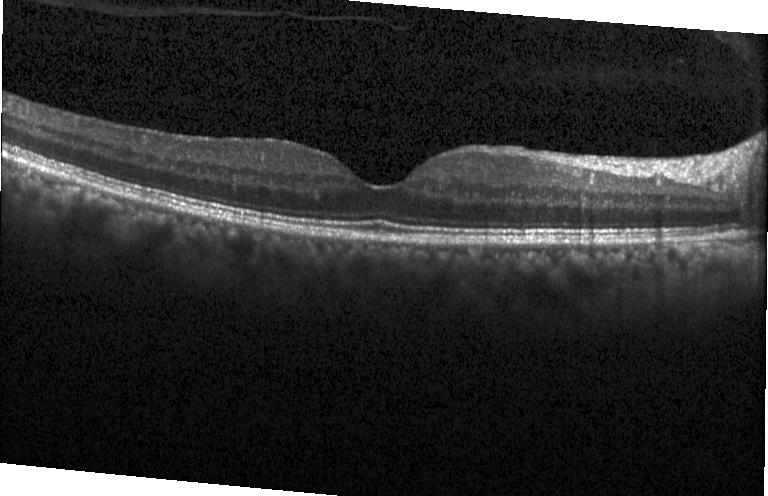
Macular OCT: no CNV, DME, or drusen.